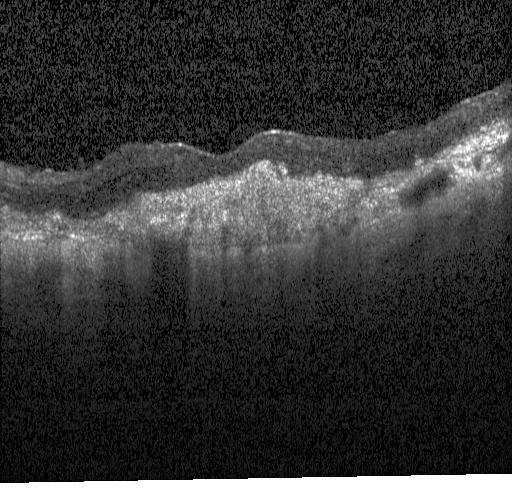
Diagnosis: choroidal neovascularization.